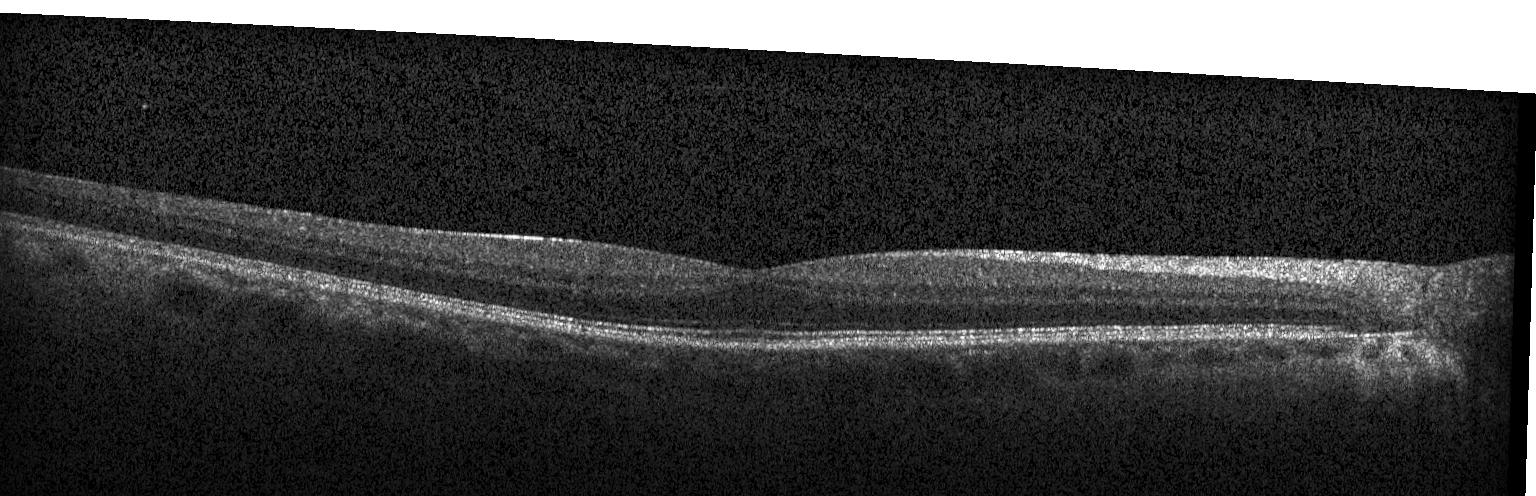

Retinal OCT cross-section; spectral-domain optical coherence tomography — The scan shows no CNV, DME, or drusen.